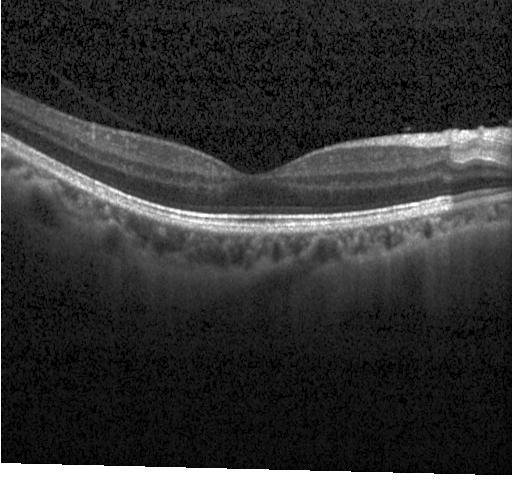 Finding: no CNV, no DME, and no drusen.